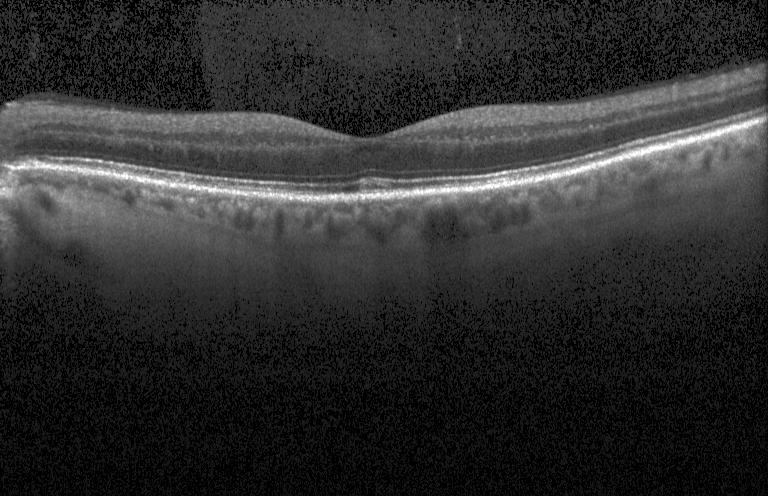
Optical coherence tomography scan; spectral-domain optical coherence tomography; acquired on a Heidelberg Spectralis; fovea-centered
Impression: no choroidal neovascularization, diabetic macular edema, or drusen.